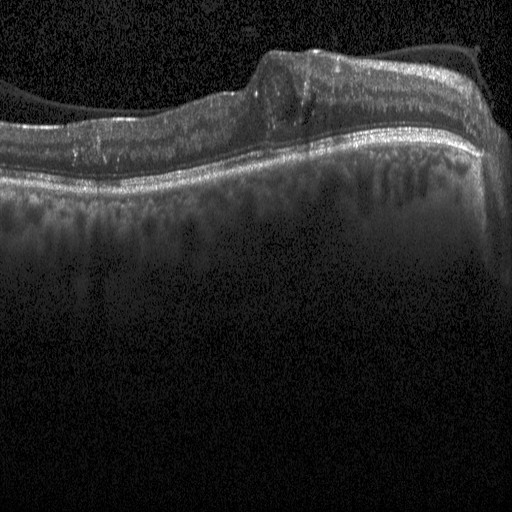

Acquired on a Heidelberg Spectralis, spectral-domain OCT, OCT B-scan
The scan shows diabetic macular edema (DME).